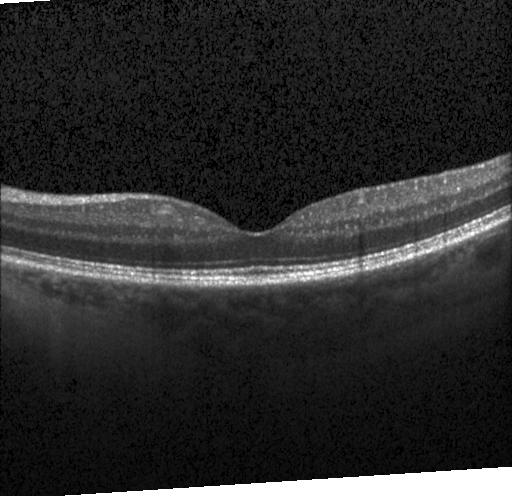
OCT line scan. Macular OCT: neither choroidal neovascularization, diabetic macular edema, nor drusen.